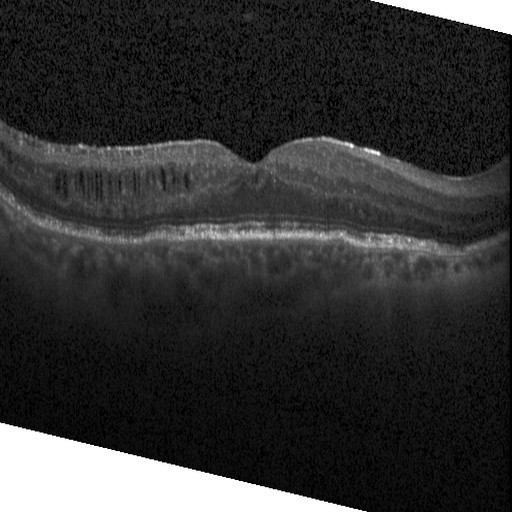
Retinal OCT cross-section showing diabetic macular edema.